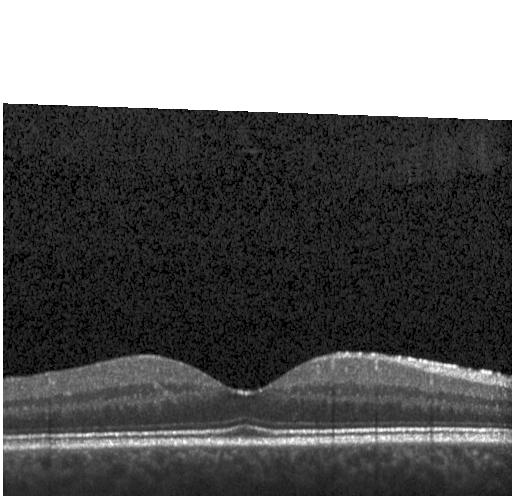
Retinal OCT cross-section showing neither choroidal neovascularization, diabetic macular edema, nor drusen.